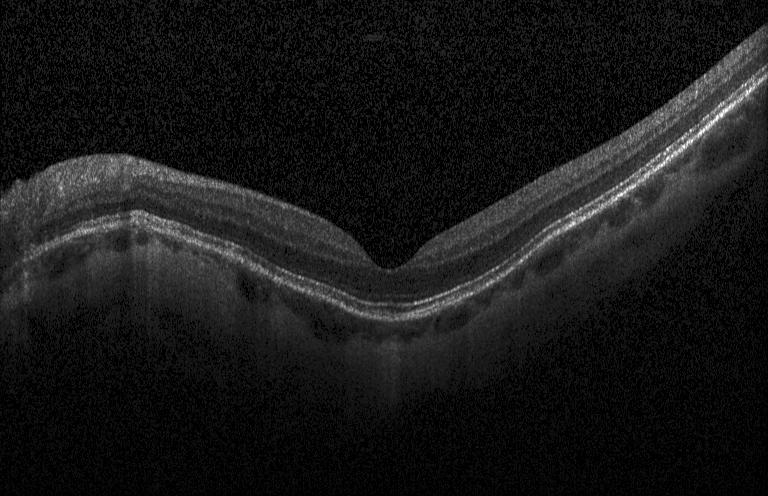
Through the macula; spectral-domain OCT; OCT B-scan.
Finding: no CNV, no DME, and no drusen.